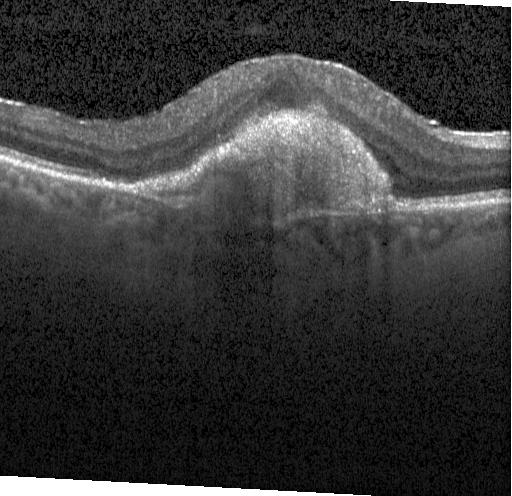
Macular OCT demonstrating CNV.